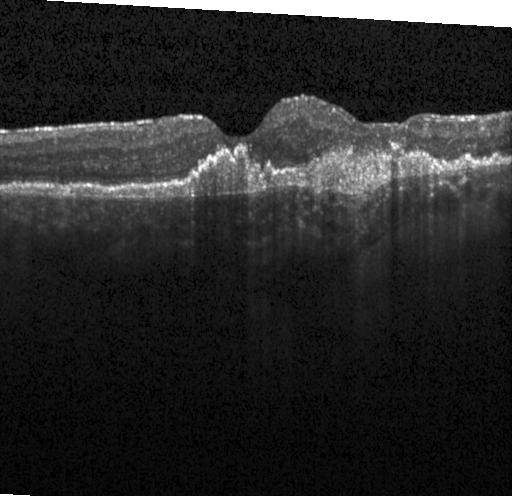 Retinal OCT B-scan — Assessment: choroidal neovascularization.